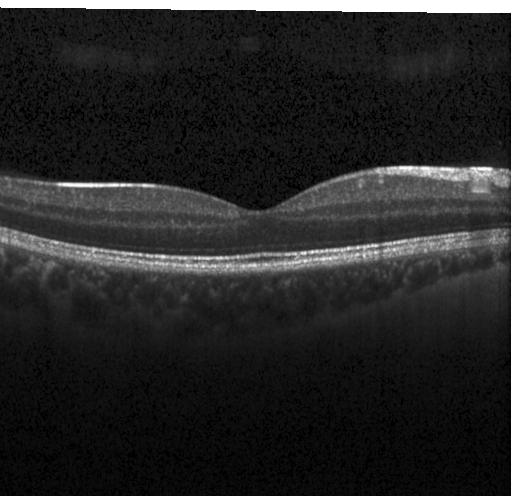
Spectral-domain optical coherence tomography, retinal OCT B-scan
Diagnosis: no evidence of CNV, DME, or drusen.